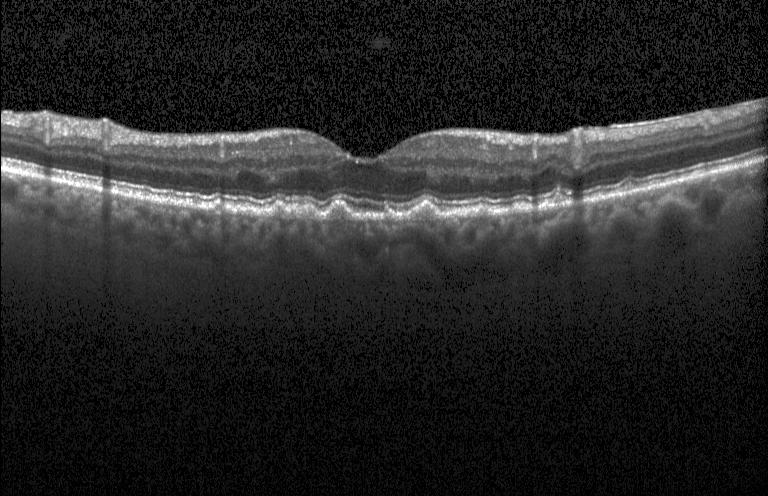 Optical coherence tomography B-scan. Finding: sub-RPE drusenoid deposits.